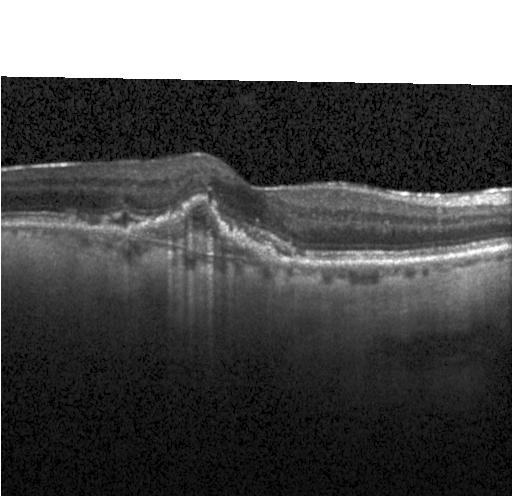 Retinal OCT cross-section
Diagnosis: a choroidal neovascular membrane.